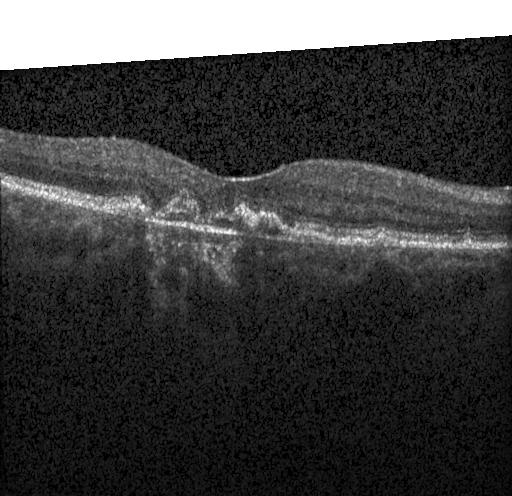

Diagnosis: choroidal neovascularization.